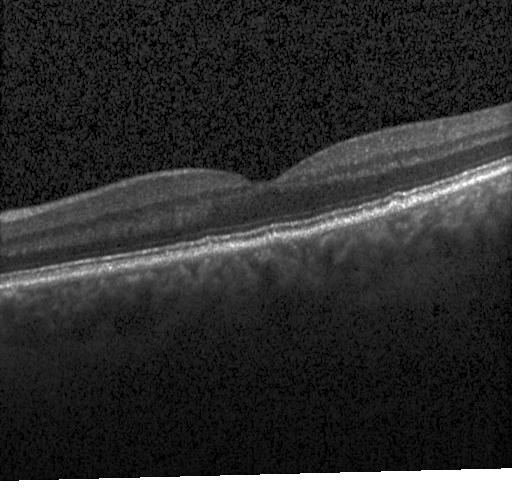 OCT line scan · Heidelberg Spectralis OCT system · centered on the fovea.
Assessment: multiple drusen.